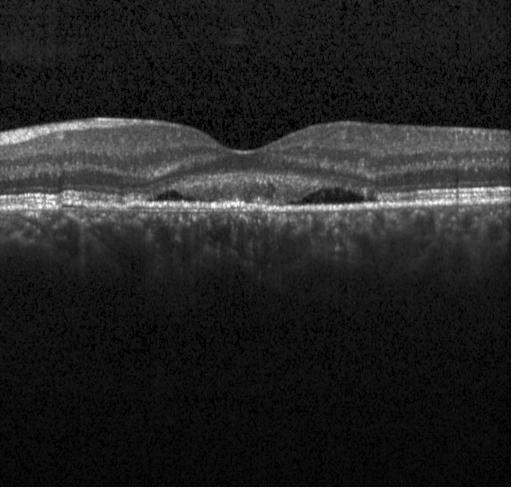

Retinal OCT B-scan · spectral-domain OCT.
Macular OCT: choroidal neovascularization (CNV).